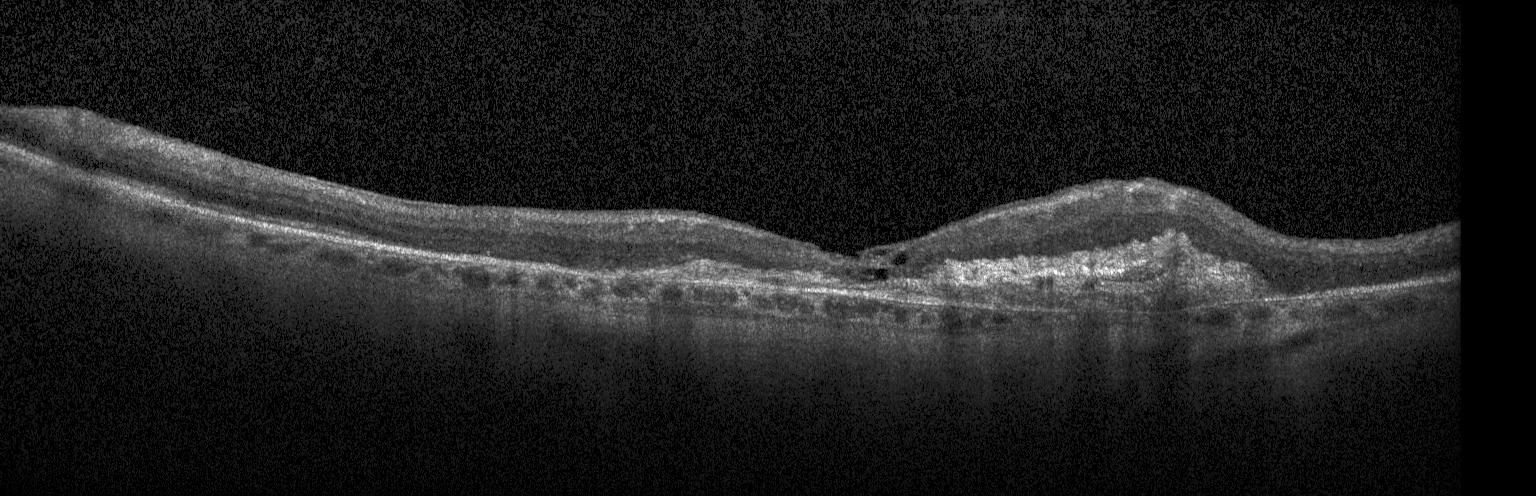 Diagnosis: choroidal neovascularization (CNV).